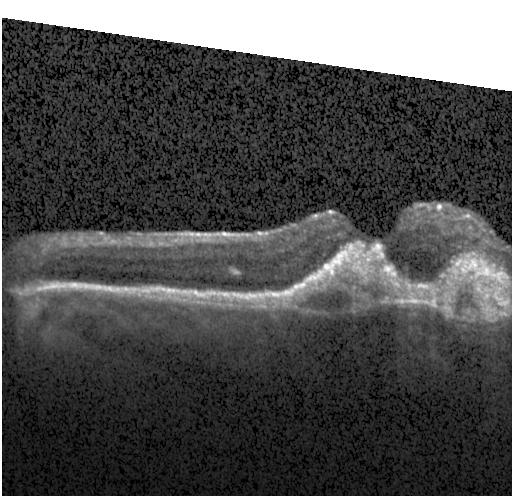 Macular OCT: choroidal neovascularization (CNV).